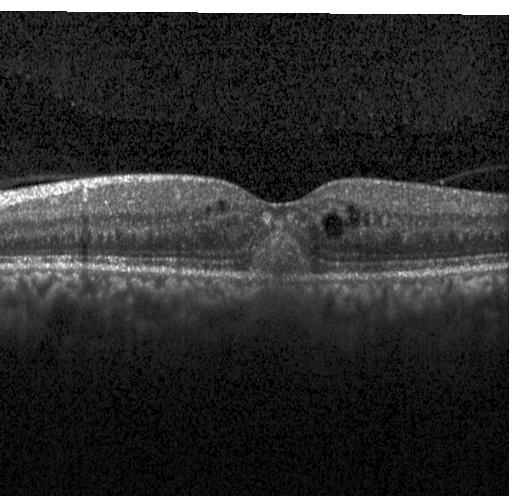

Choroidal neovascularization (CNV).